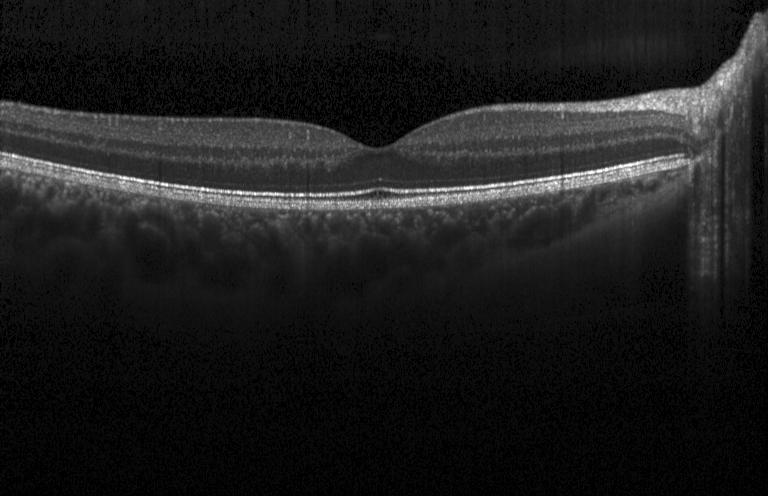 Through the macula; acquired on a Heidelberg Spectralis; SD-OCT; retinal OCT B-scan. Dx: neither choroidal neovascularization, diabetic macular edema, nor drusen.